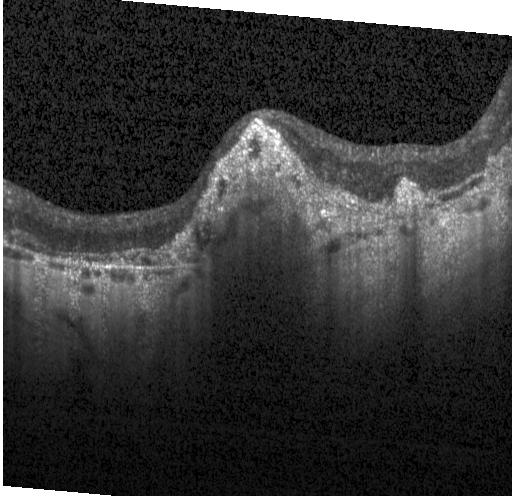

Macular scan · retinal OCT B-scan. Impression: a choroidal neovascular membrane.